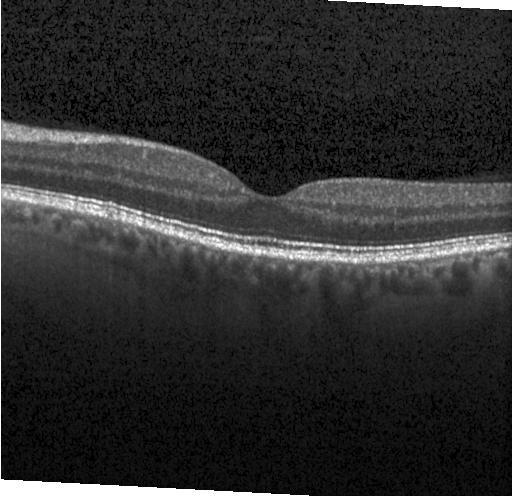 Acquired on a Heidelberg Spectralis · OCT B-scan.
Diagnosis: no choroidal neovascularization, diabetic macular edema, or drusen.